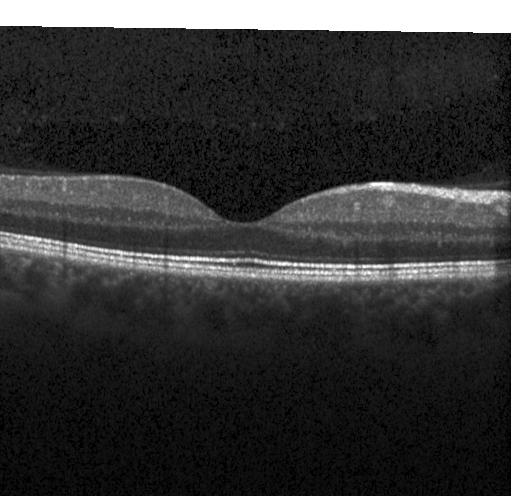
Retinal OCT cross-section.
No CNV, DME, or drusen.